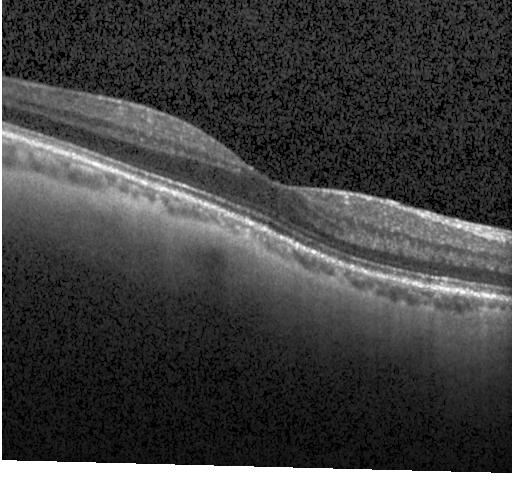

Finding: no choroidal neovascularization, no diabetic macular edema, and no drusen.